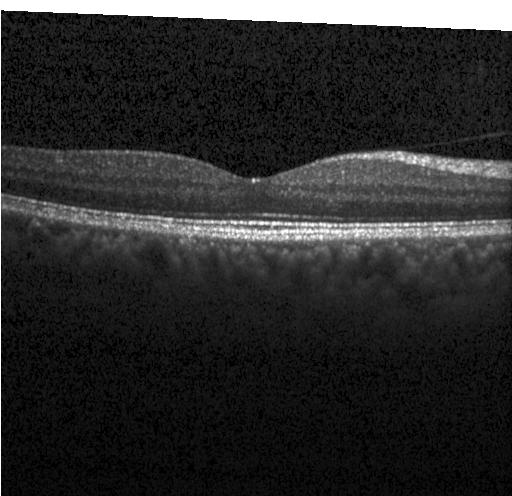 SD-OCT · optical coherence tomography scan · Heidelberg Spectralis · fovea-centered. Finding: no choroidal neovascularization, no diabetic macular edema, and no drusen.